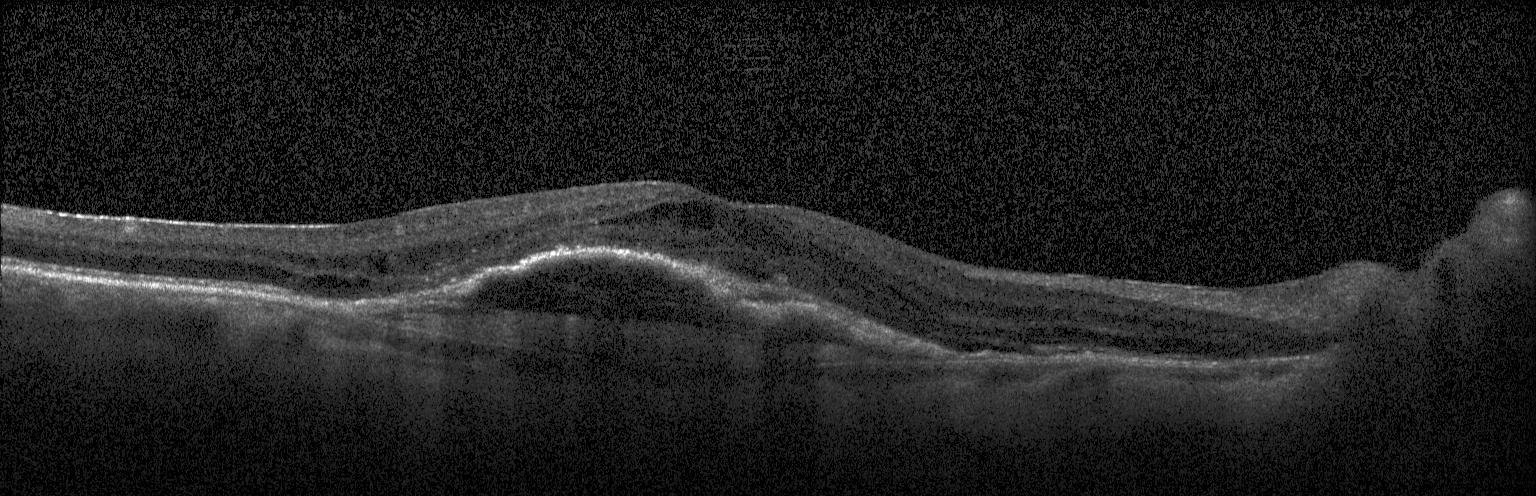

Macular OCT: a choroidal neovascular membrane.